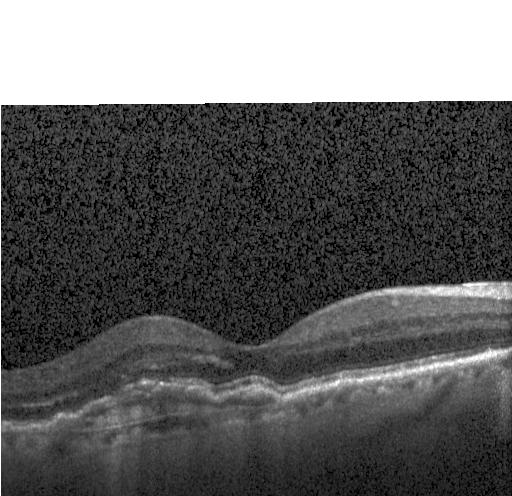 Spectral-domain OCT · optical coherence tomography B-scan · Heidelberg Spectralis
Diagnosis: a choroidal neovascular membrane.